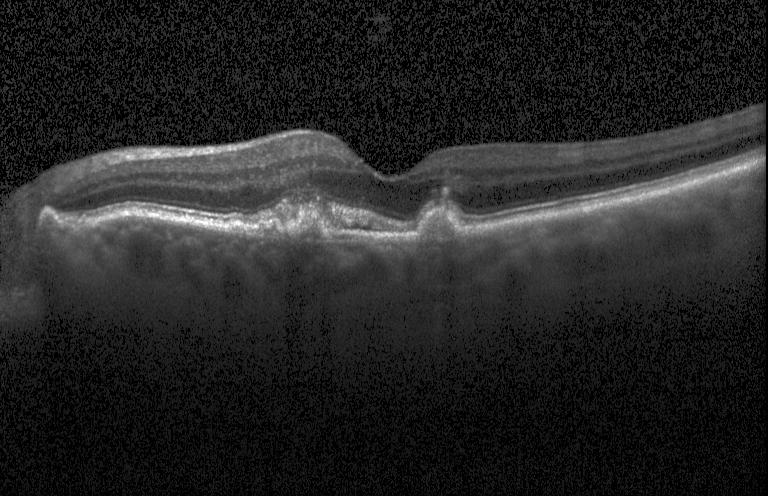 Centered on the fovea. OCT line scan.
Finding: a choroidal neovascular membrane.